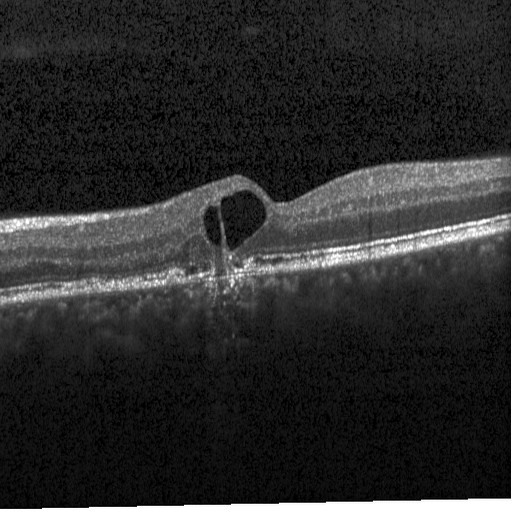
OCT line scan
Dx: diabetic macular edema (DME).